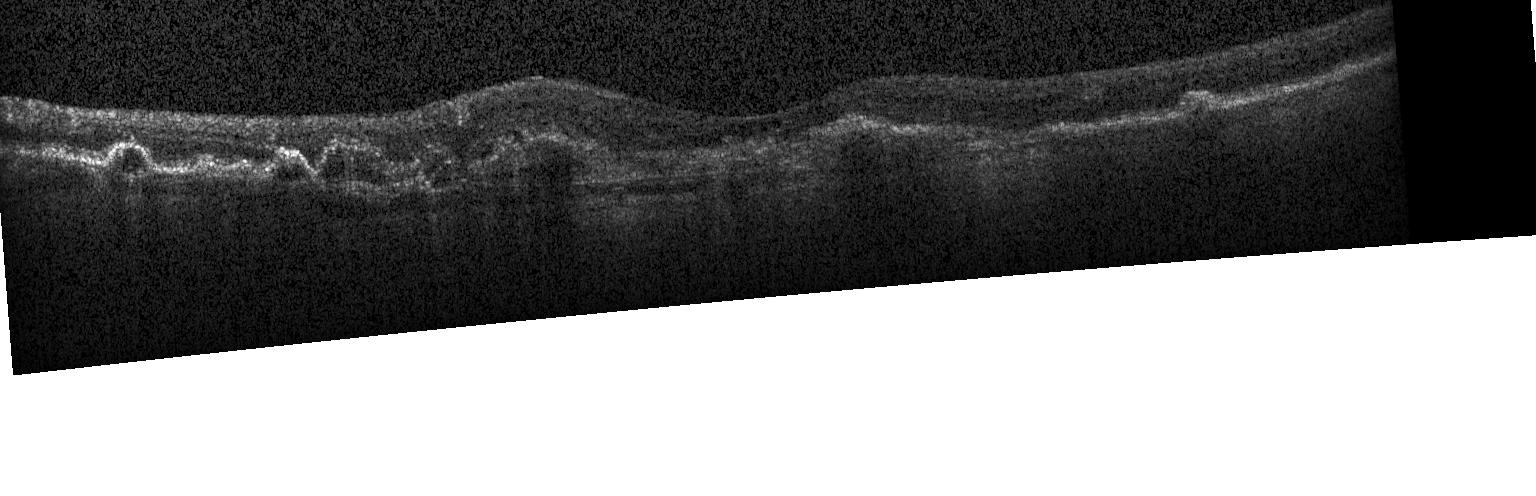 The scan shows a choroidal neovascular membrane.